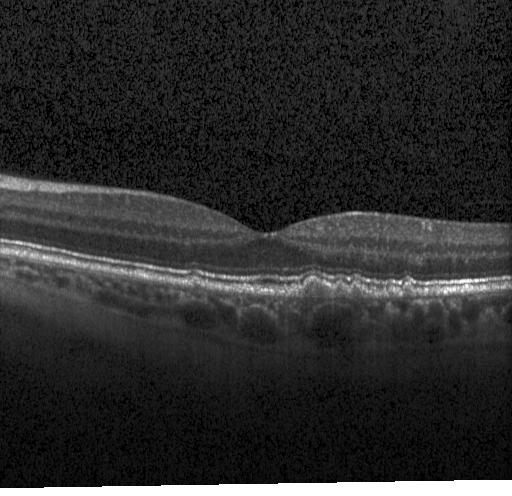

Optical coherence tomography B-scan · horizontal scan through the fovea · instrument: Heidelberg Spectralis · spectral-domain optical coherence tomography.
Dx: drusen.